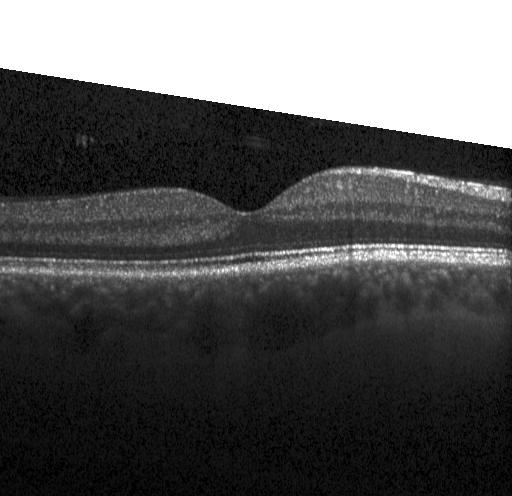
Optical coherence tomography B-scan; spectral-domain optical coherence tomography; macular scan; instrument: Heidelberg Spectralis
Impression: no evidence of choroidal neovascularization, diabetic macular edema, or drusen.